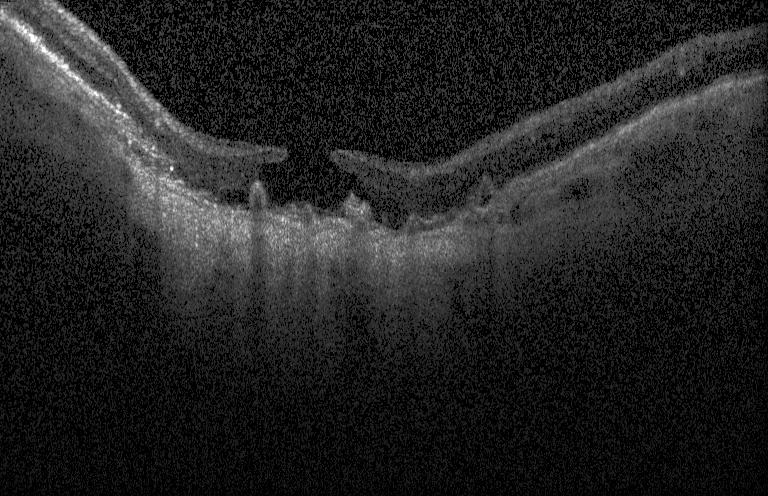 OCT line scan · spectral-domain OCT
Finding: a choroidal neovascular membrane.